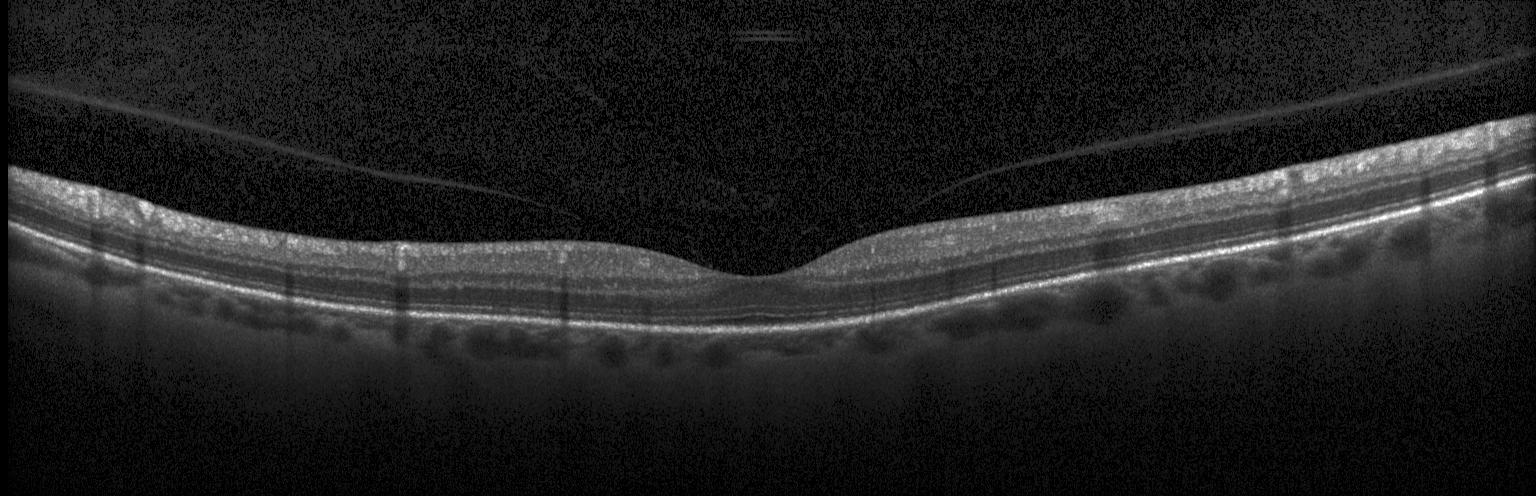

Spectral-domain OCT · retinal OCT cross-section · fovea-centered.
Dx: no CNV, no DME, and no drusen.